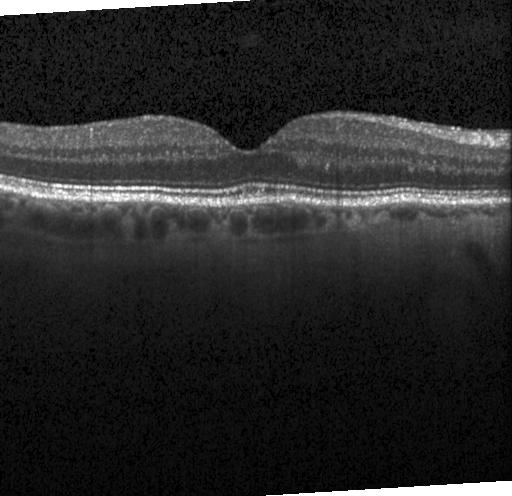 Retinal OCT B-scan — Finding: no evidence of CNV, DME, or drusen.